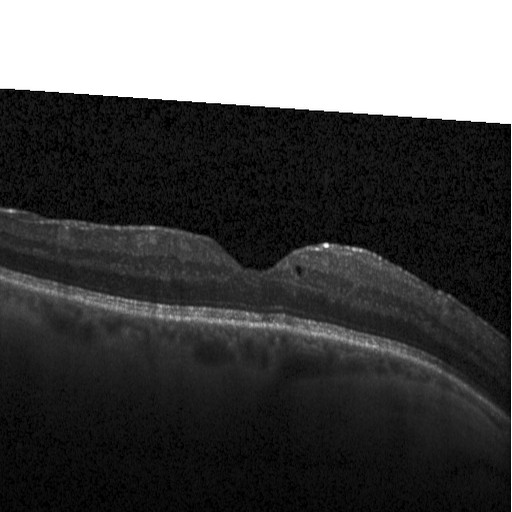
Macular scan; SD-OCT; acquired on a Heidelberg Spectralis; retinal OCT cross-section — OCT finding: DME.